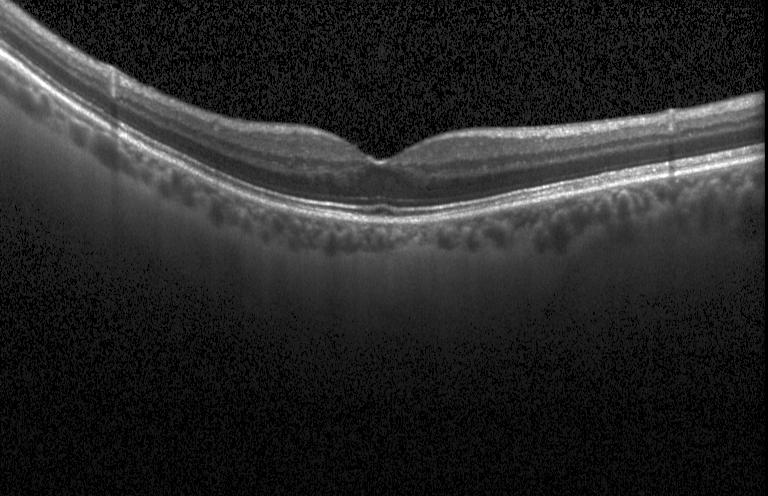
Optical coherence tomography scan
Finding: no evidence of CNV, DME, or drusen.